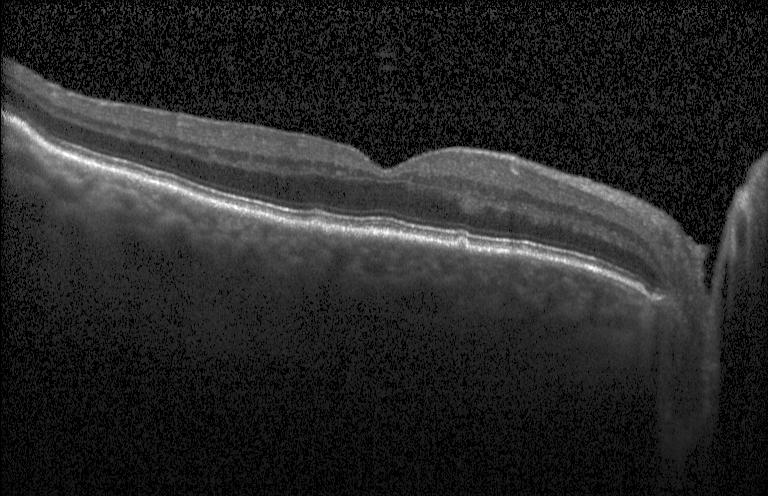 Retinal OCT B-scan · acquired on a Heidelberg Spectralis — The scan shows multiple drusen.